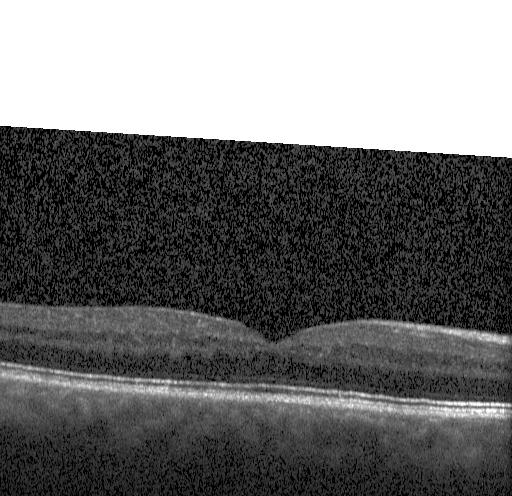

Heidelberg Spectralis, OCT line scan, spectral-domain optical coherence tomography. Macular OCT: no choroidal neovascularization, diabetic macular edema, or drusen.